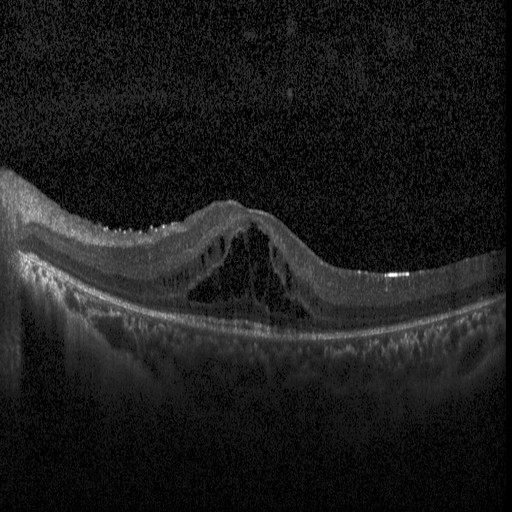

Horizontal scan through the fovea; spectral-domain OCT; Heidelberg Spectralis; retinal OCT B-scan
Finding: DME.